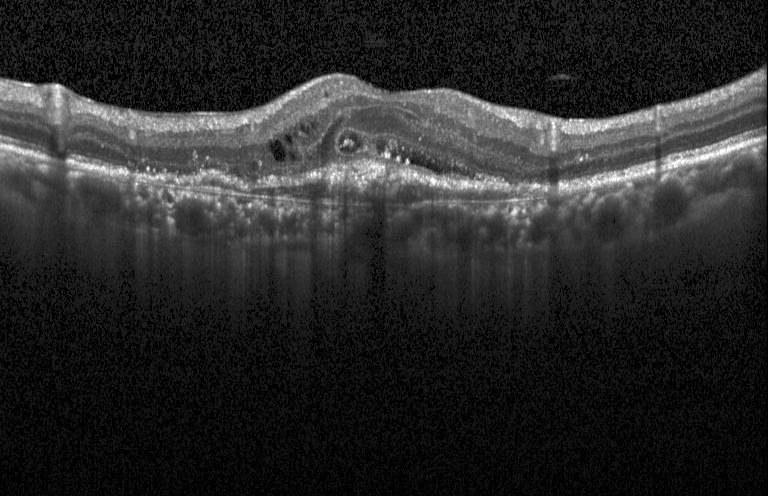 Impression: choroidal neovascularization.